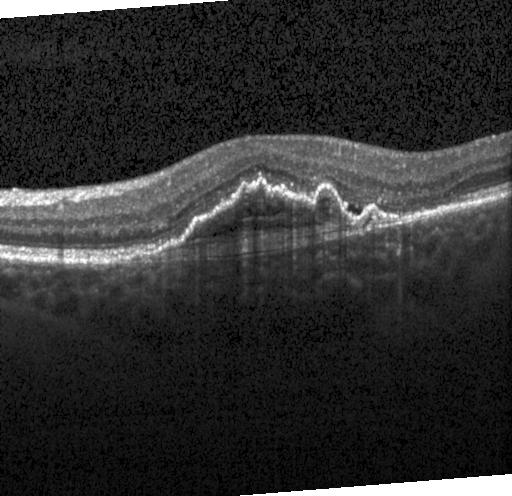

Optical coherence tomography scan
Macular OCT: a choroidal neovascular membrane.